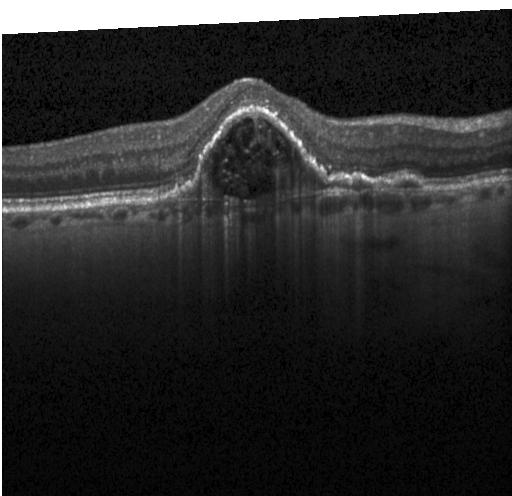 Dx: a choroidal neovascular membrane.